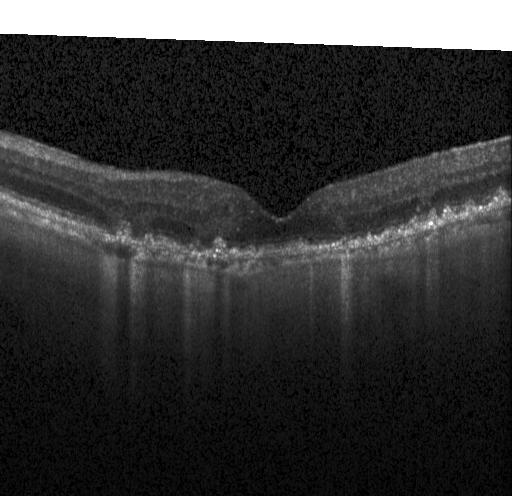 SD-OCT; centered on the fovea; instrument: Heidelberg Spectralis; OCT line scan — Diagnosis: a choroidal neovascular membrane.